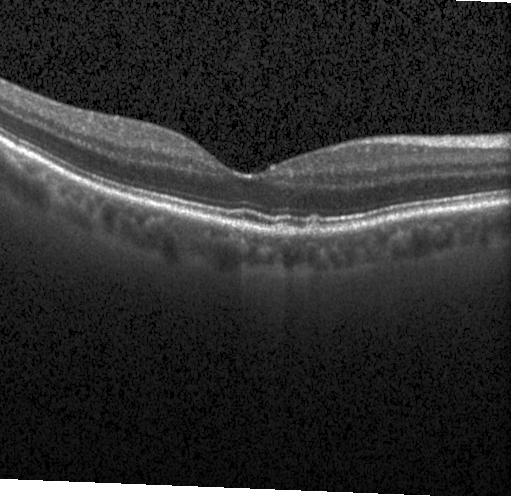 Through the macula · optical coherence tomography B-scan. Sub-RPE drusenoid deposits.